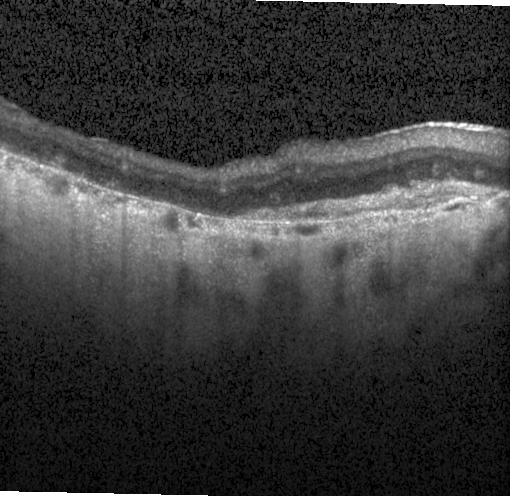

CNV.